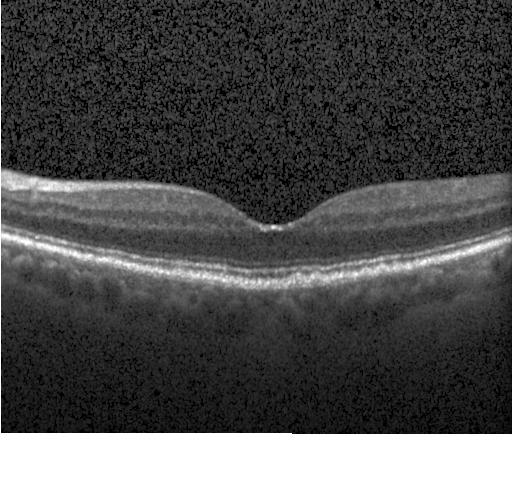 Optical coherence tomography B-scan; macular scan; spectral-domain optical coherence tomography.
Macular OCT: multiple drusen.